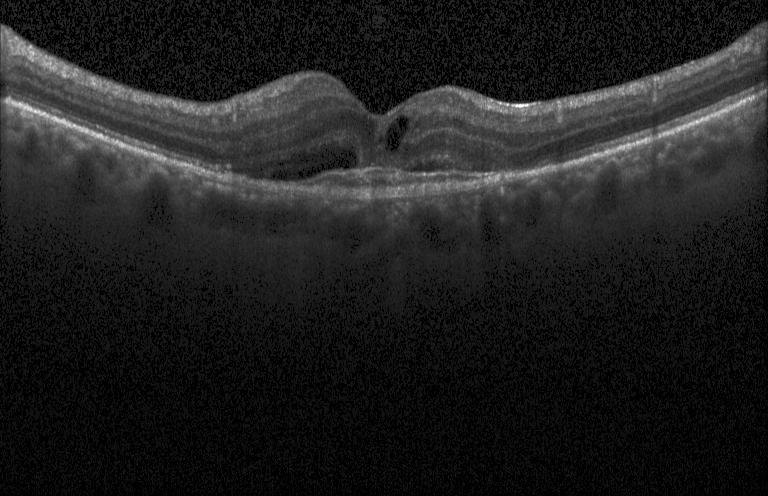

OCT line scan · Heidelberg Spectralis OCT system. A choroidal neovascular membrane.